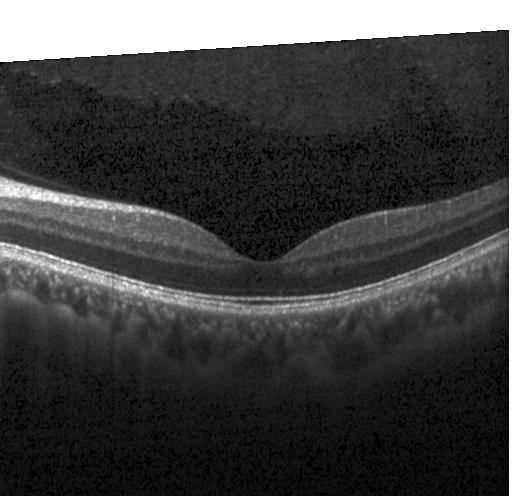

SD-OCT; optical coherence tomography B-scan; fovea-centered.
Diagnosis: no choroidal neovascularization, diabetic macular edema, or drusen.